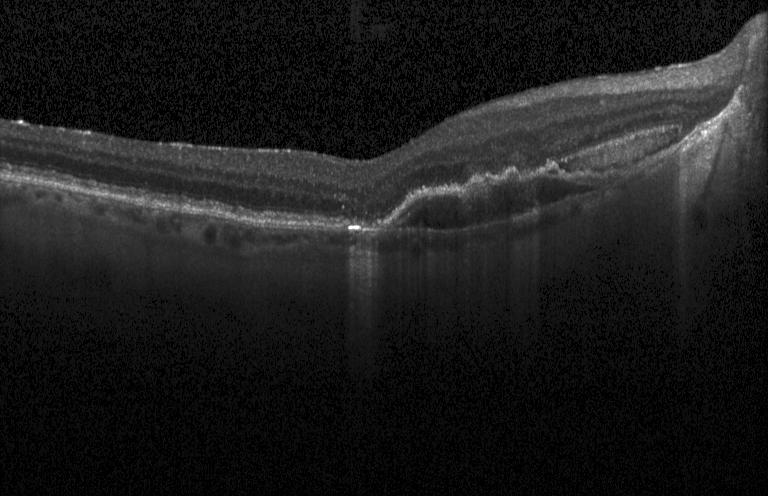

Finding: choroidal neovascularization (CNV).